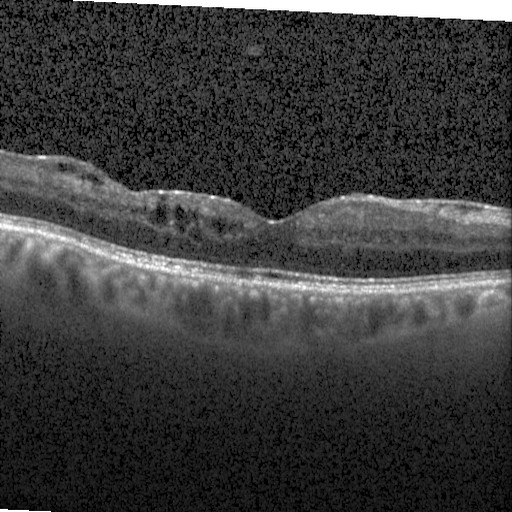 OCT line scan, SD-OCT, Heidelberg Spectralis.
Diagnosis: DME.